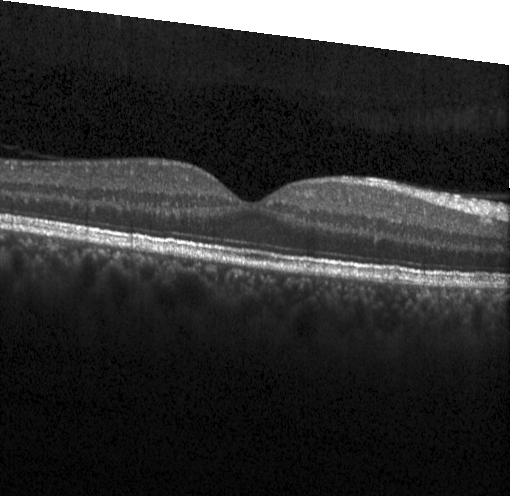
Centered on the fovea; OCT line scan. No evidence of choroidal neovascularization, diabetic macular edema, or drusen.